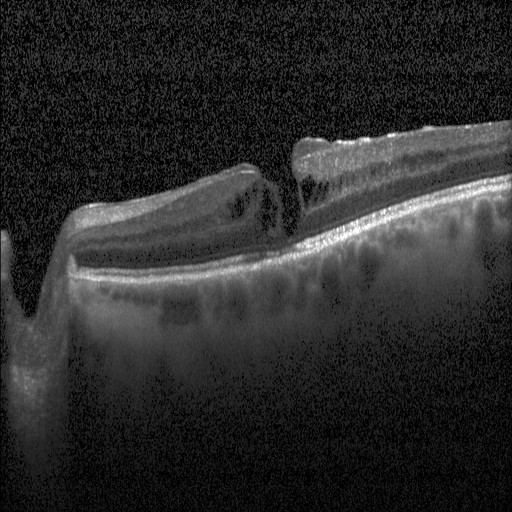

Retinal OCT cross-section.
Diagnosis: diabetic macular edema.